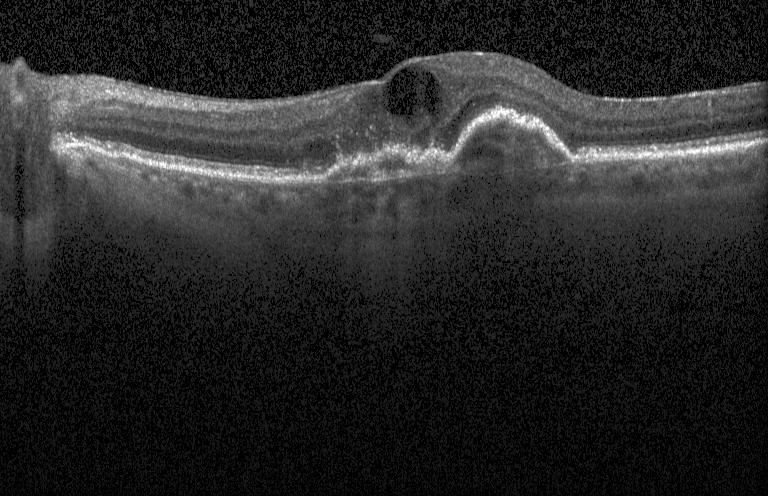

Retinal OCT B-scan · horizontal scan through the fovea · spectral-domain OCT · instrument: Heidelberg Spectralis
Assessment: CNV.